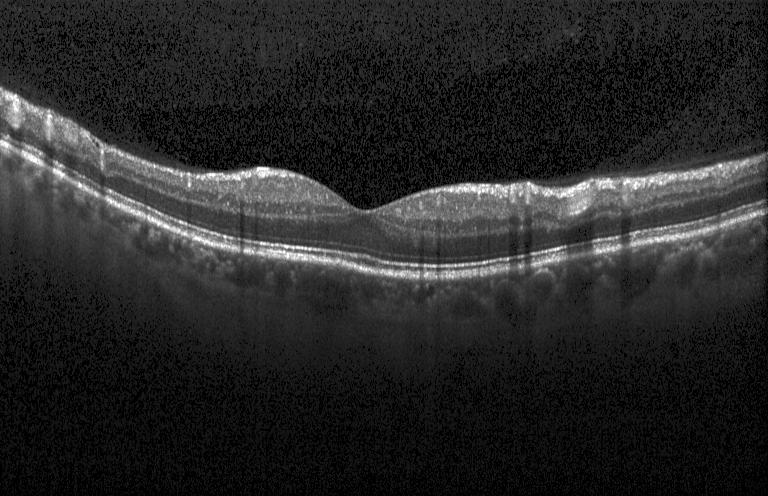 Macular OCT demonstrating no evidence of choroidal neovascularization, diabetic macular edema, or drusen.